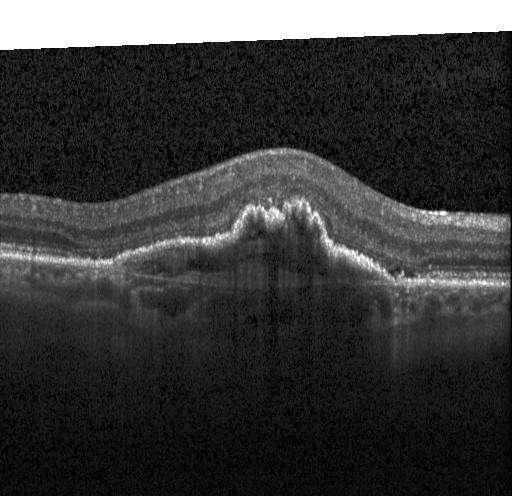 Instrument: Heidelberg Spectralis, macular scan, SD-OCT, OCT B-scan
Diagnosis: a choroidal neovascular membrane.